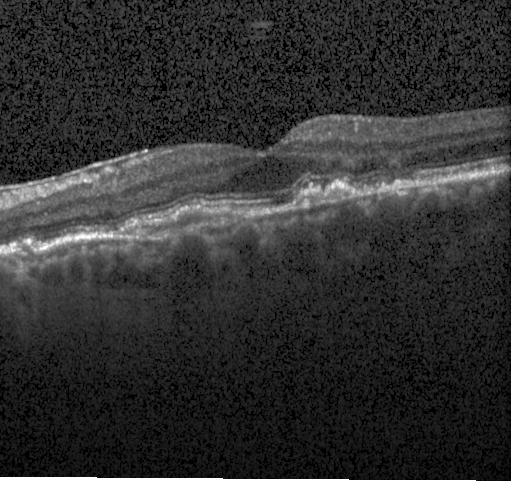 The scan shows CNV.